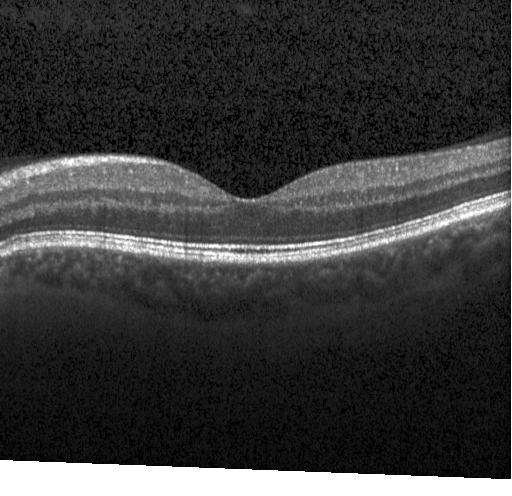
Dx: neither choroidal neovascularization, diabetic macular edema, nor drusen.